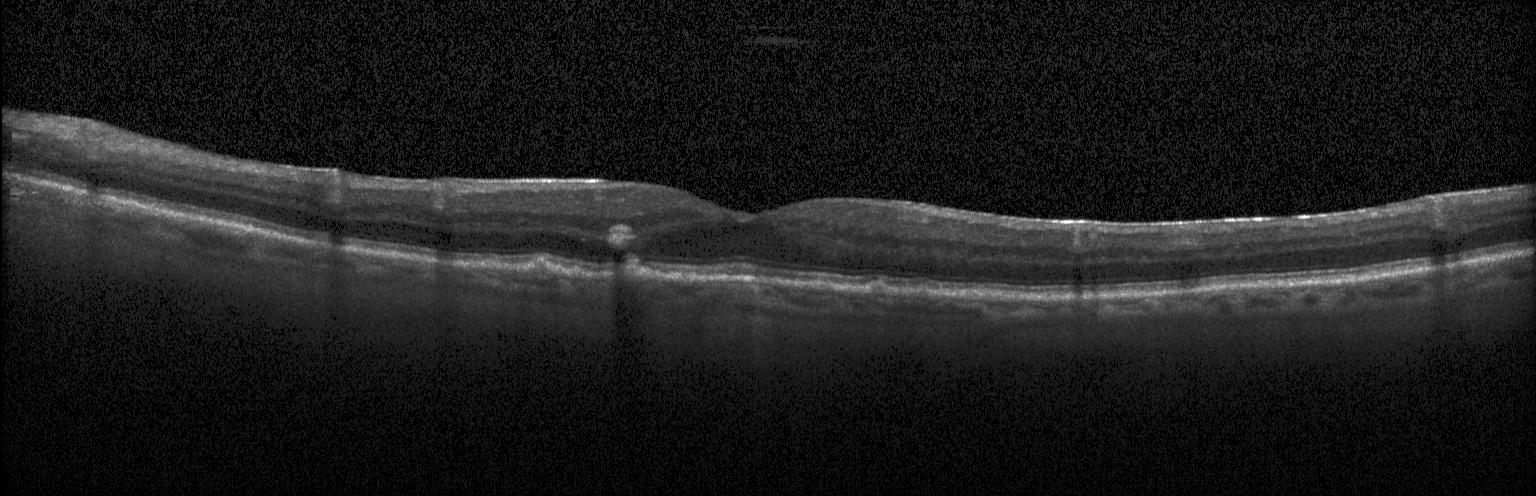 Optical coherence tomography B-scan.
Macular OCT: multiple drusen.